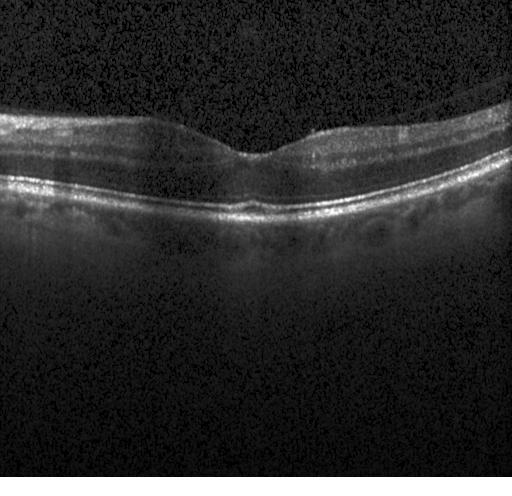 OCT line scan. Dx: no choroidal neovascularization, diabetic macular edema, or drusen.